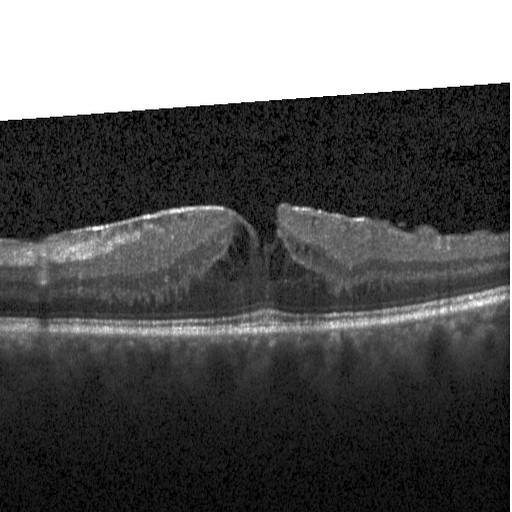 Retinal OCT cross-section · Heidelberg Spectralis OCT system.
Diagnosis: DME.